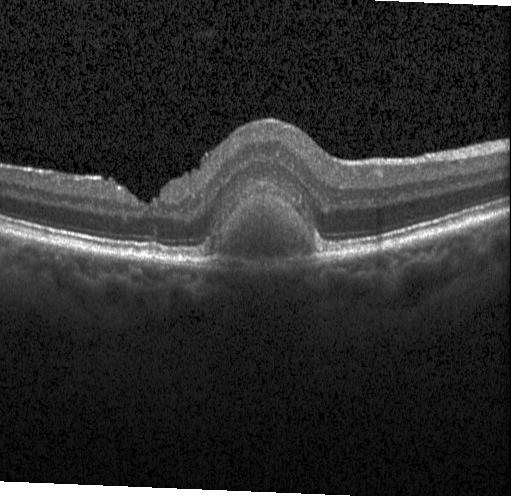

Optical coherence tomography B-scan.
The scan shows CNV.